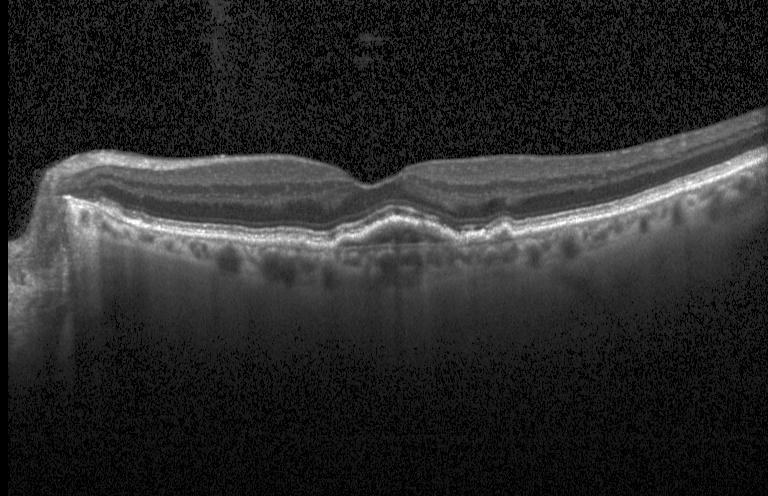

Optical coherence tomography B-scan · instrument: Heidelberg Spectralis
CNV.